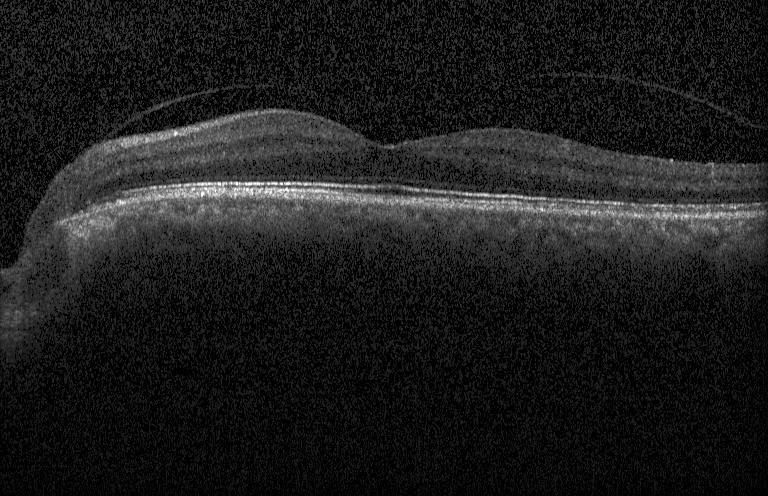

Dx: neither choroidal neovascularization, diabetic macular edema, nor drusen.